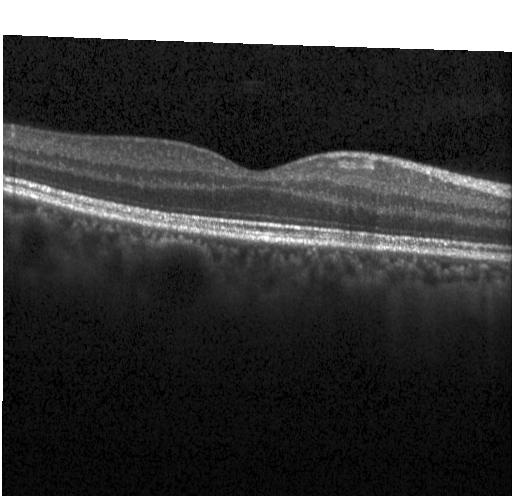 Finding: no choroidal neovascularization, no diabetic macular edema, and no drusen.